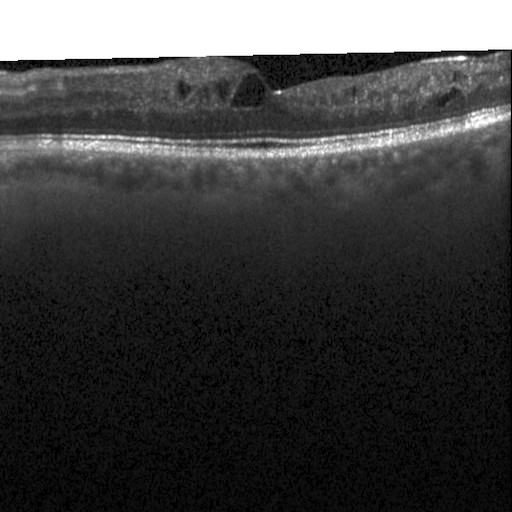 OCT finding: DME.